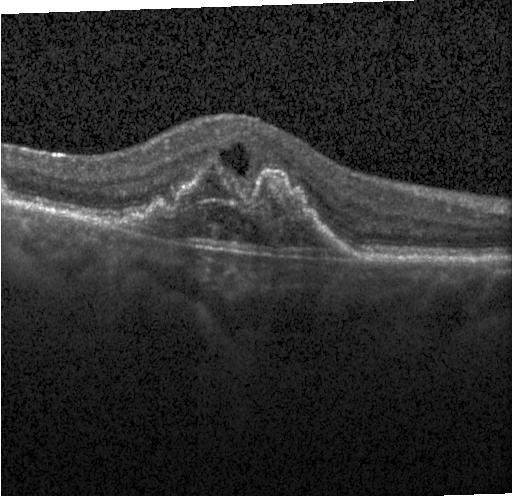 Horizontal scan through the fovea · Heidelberg Spectralis OCT system · OCT B-scan — Impression: a choroidal neovascular membrane.